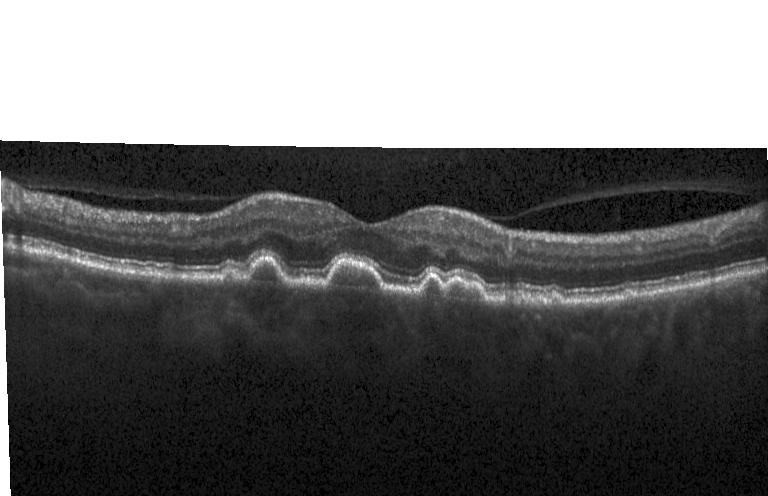

OCT scan showing multiple drusen.